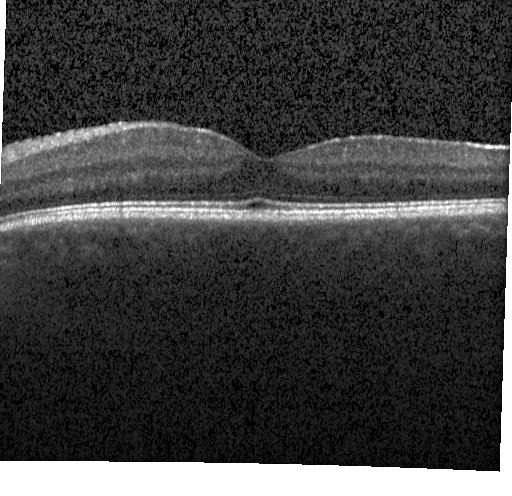
Optical coherence tomography B-scan — Assessment: no choroidal neovascularization, diabetic macular edema, or drusen.